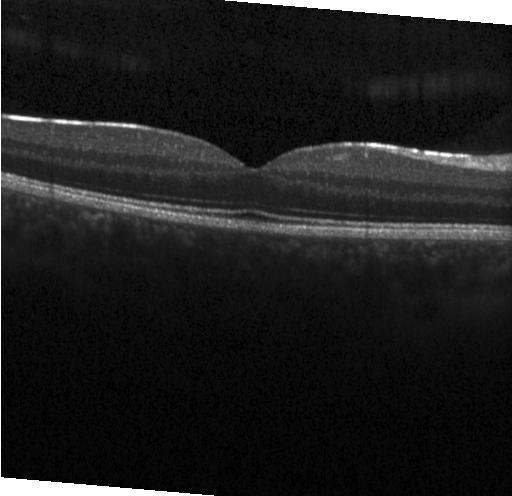

Spectral-domain OCT, OCT B-scan, fovea-centered.
Macular OCT: neither CNV, DME, nor drusen.